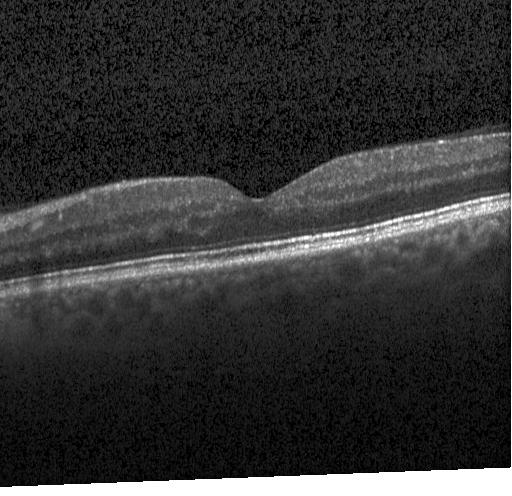 OCT finding: no choroidal neovascularization, no diabetic macular edema, and no drusen.